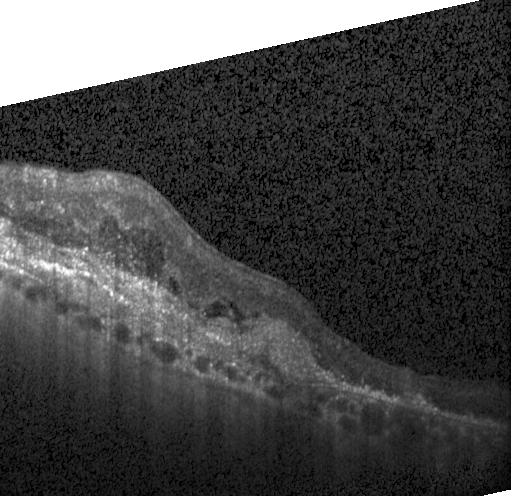 Centered on the fovea · retinal OCT B-scan — Finding: choroidal neovascularization.